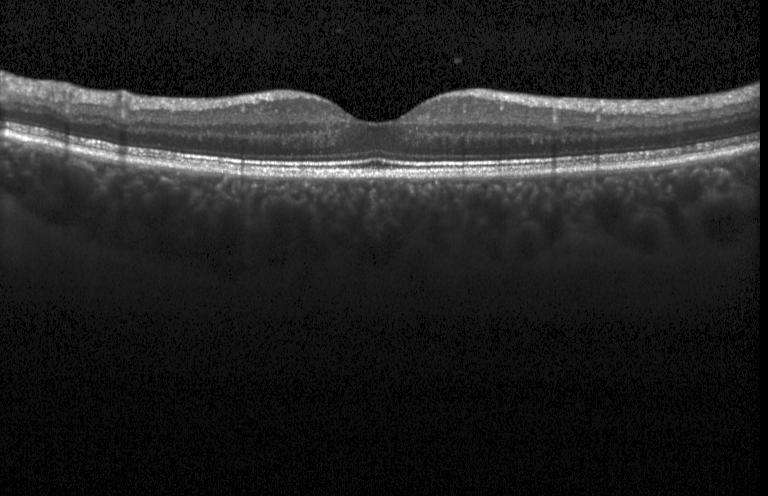 Diagnosis: no evidence of choroidal neovascularization, diabetic macular edema, or drusen.